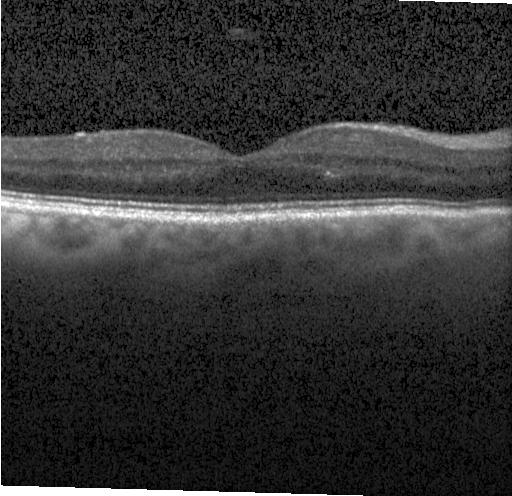
Spectral-domain OCT · OCT line scan · acquired on a Heidelberg Spectralis · through the macula
This B-scan demonstrates no CNV, no DME, and no drusen.